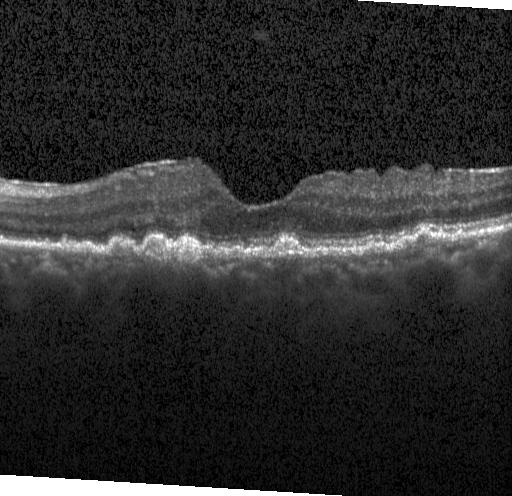 Optical coherence tomography scan, Heidelberg Spectralis OCT system.
Impression: sub-RPE drusenoid deposits.